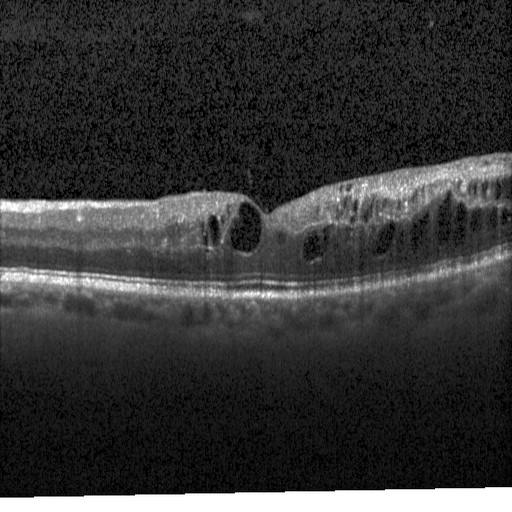
OCT B-scan
Assessment: DME.